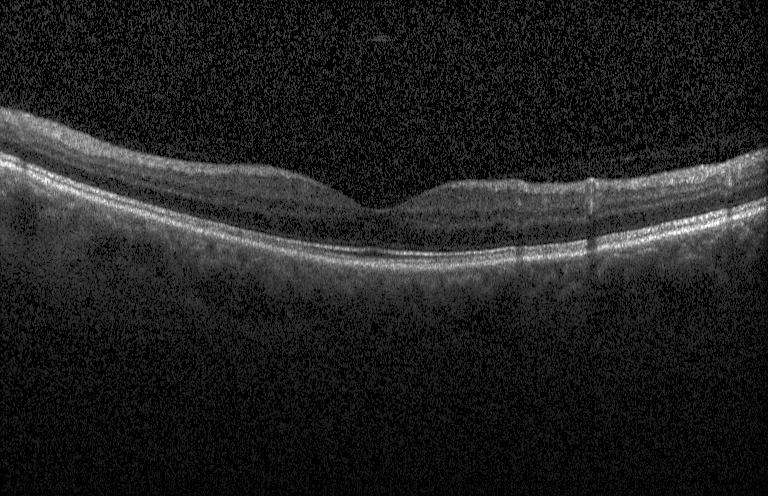 Acquired on a Heidelberg Spectralis. Retinal OCT B-scan.
Diagnosis: no evidence of choroidal neovascularization, diabetic macular edema, or drusen.